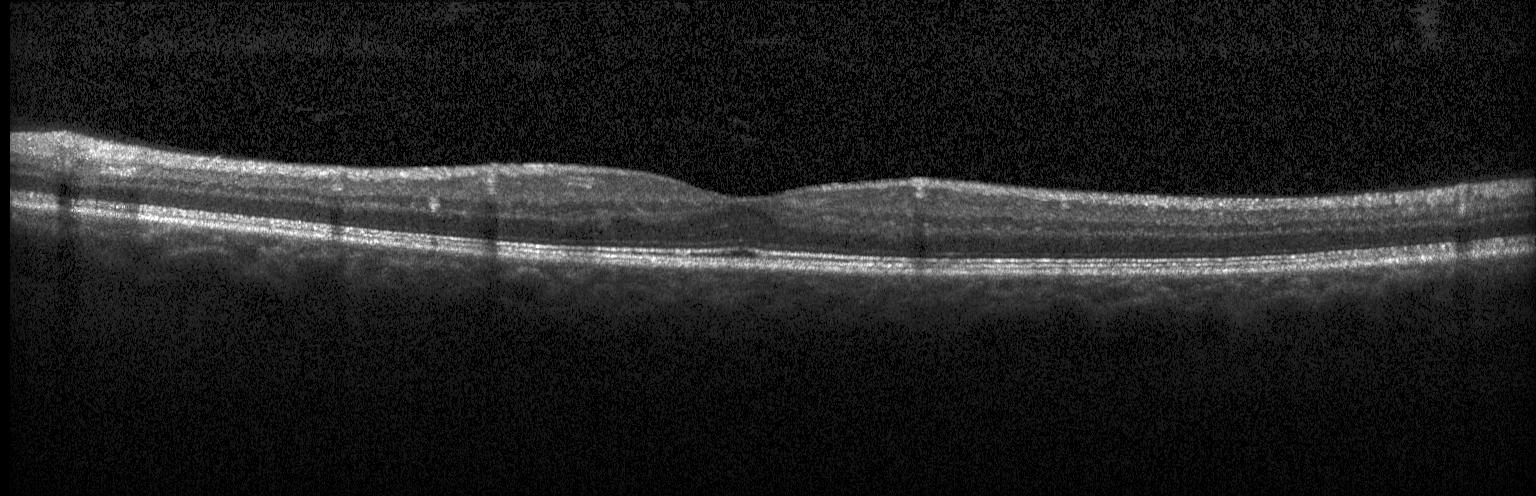 Impression: no choroidal neovascularization, diabetic macular edema, or drusen.